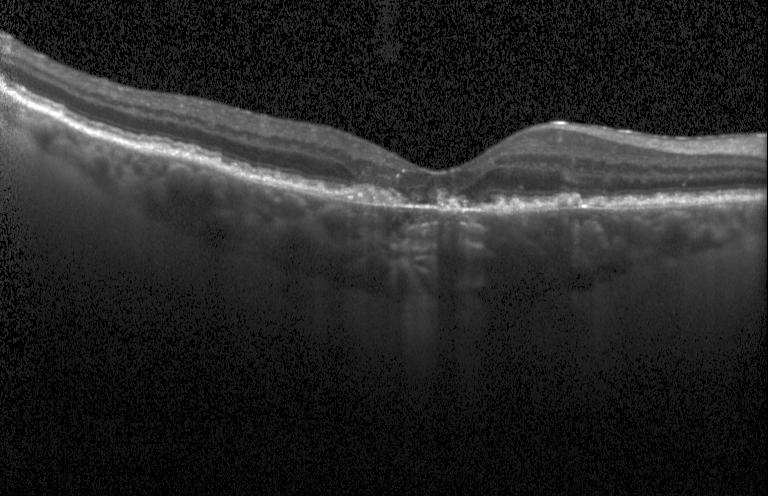

Spectral-domain OCT B-scan: a choroidal neovascular membrane.